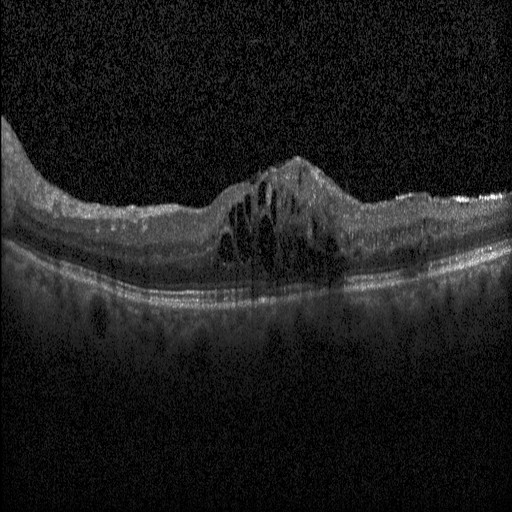 DME.